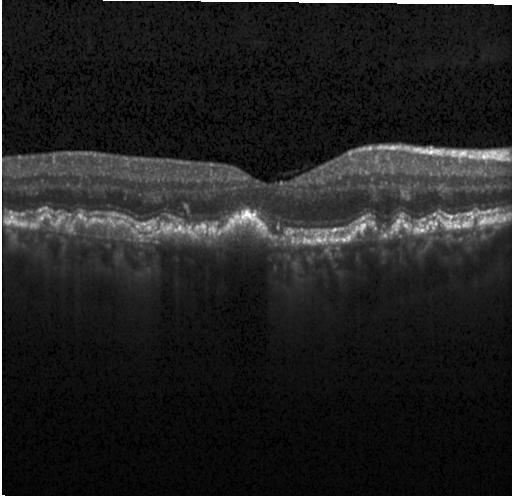 Retinal OCT cross-section showing sub-RPE drusenoid deposits.